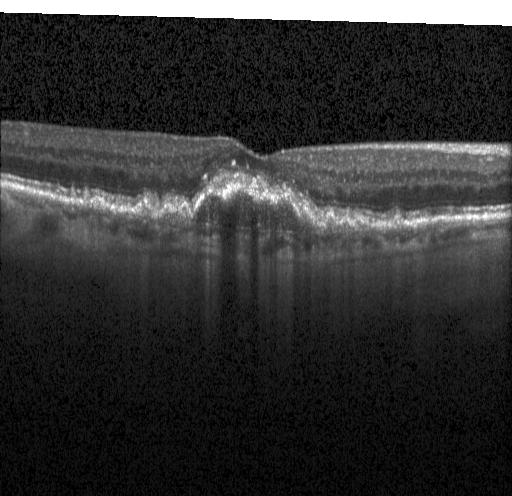
Heidelberg Spectralis OCT system. OCT B-scan. Spectral-domain optical coherence tomography. Horizontal scan through the fovea
The scan shows a choroidal neovascular membrane.